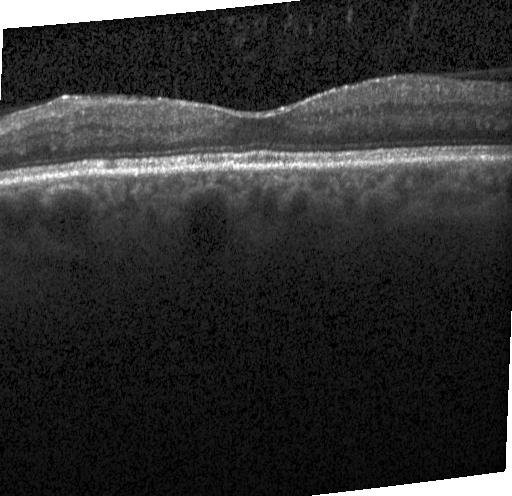
Spectral-domain OCT. Optical coherence tomography B-scan. No CNV, no DME, and no drusen.